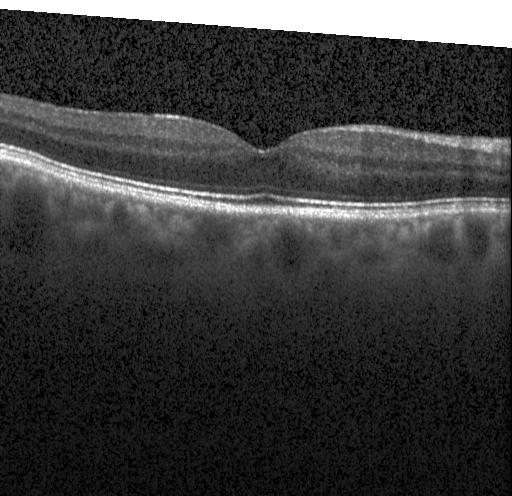
Heidelberg Spectralis, OCT line scan. The scan shows no CNV, no DME, and no drusen.